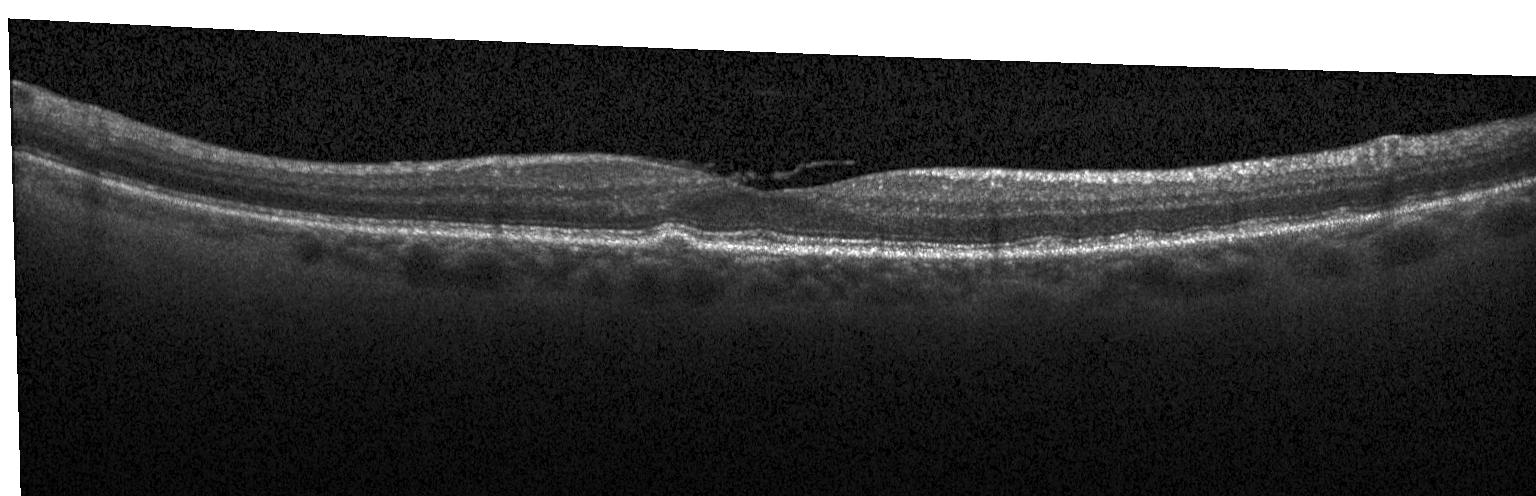

Spectral-domain OCT. Heidelberg Spectralis. Retinal OCT cross-section. Fovea-centered.
Drusen.